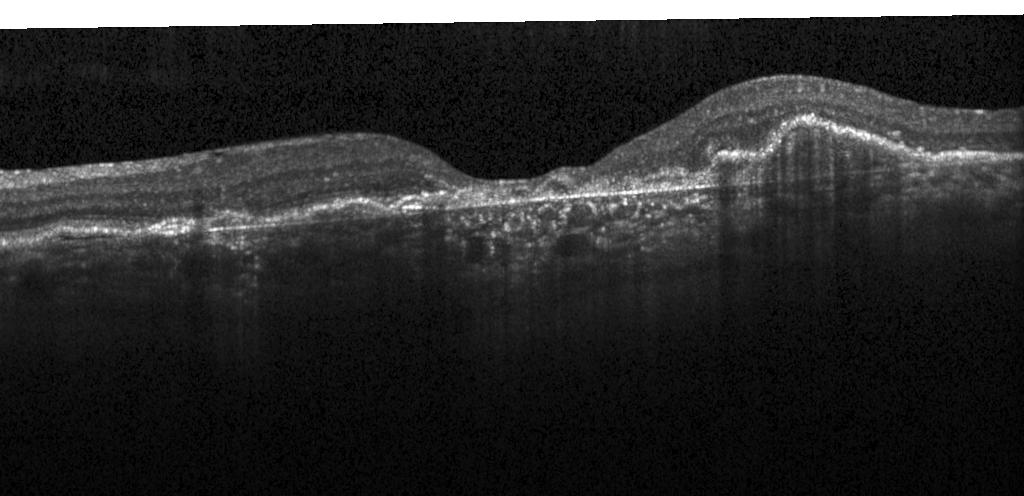
Through the macula, OCT B-scan
Impression: CNV.